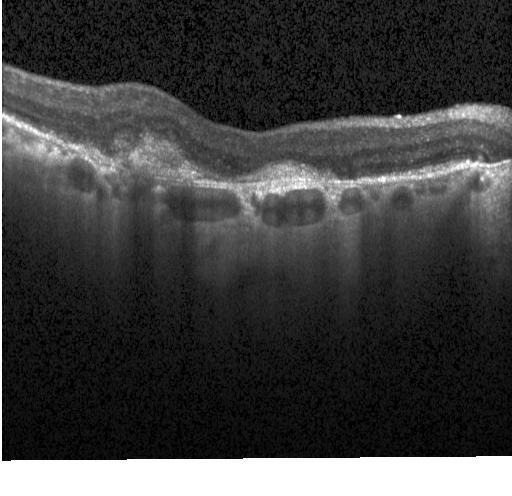

Optical coherence tomography scan.
Macular OCT: choroidal neovascularization.